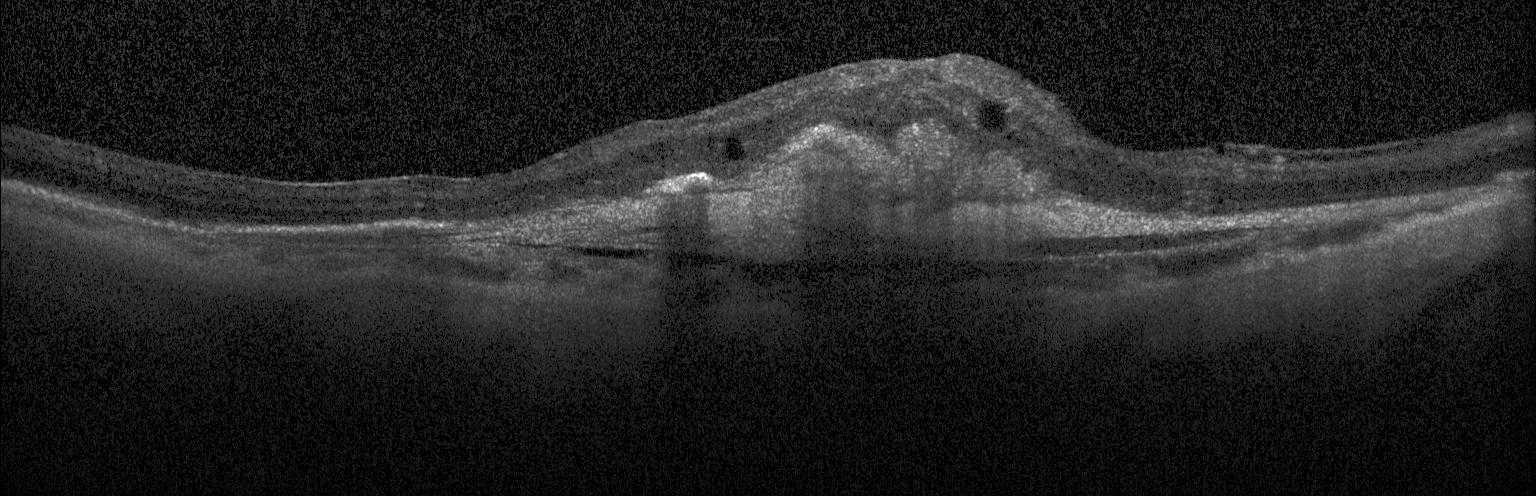

Spectral-domain optical coherence tomography. Instrument: Heidelberg Spectralis. Retinal OCT cross-section
OCT finding: choroidal neovascularization.